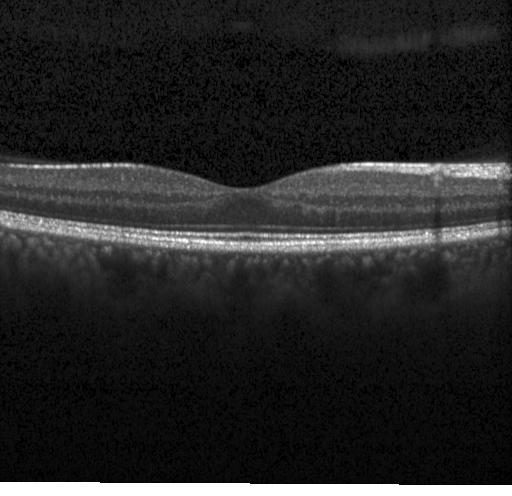 Finding: no CNV, DME, or drusen.